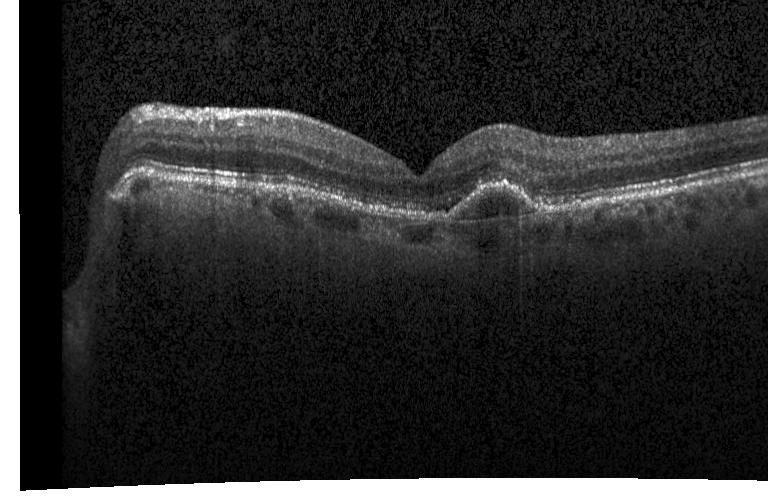 Heidelberg Spectralis, optical coherence tomography B-scan, SD-OCT, through the macula. This B-scan demonstrates choroidal neovascularization.